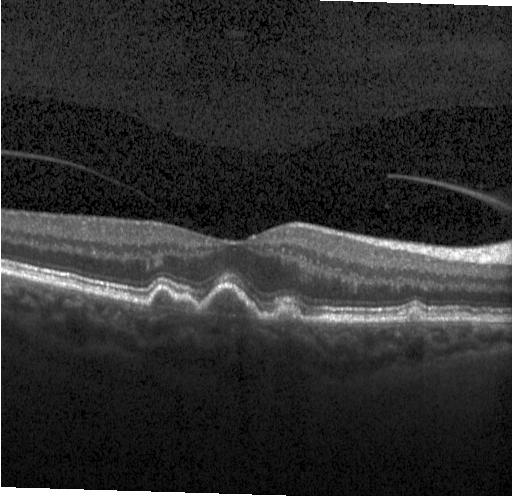
Diagnosis: CNV.